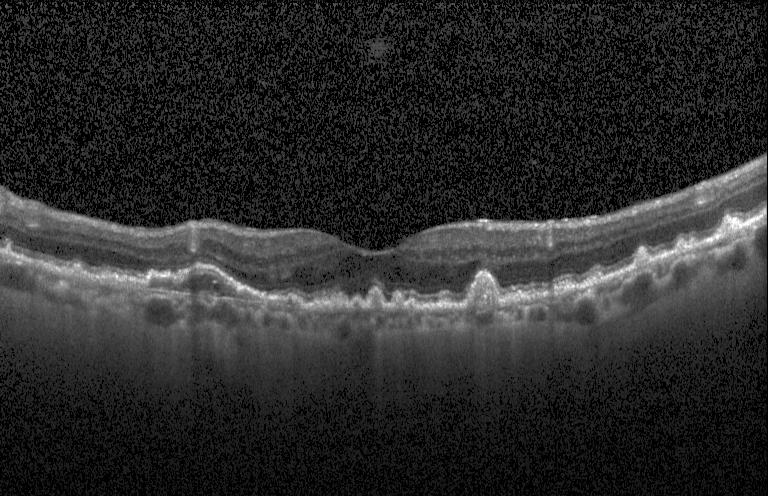

Spectral-domain OCT B-scan: multiple drusen.